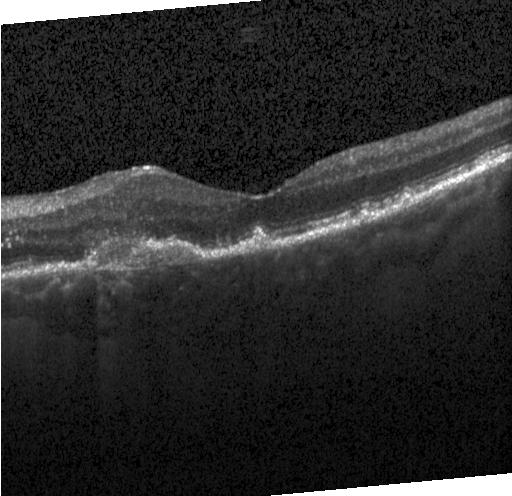 Retinal OCT B-scan. Spectral-domain OCT. Instrument: Heidelberg Spectralis. Impression: a choroidal neovascular membrane.